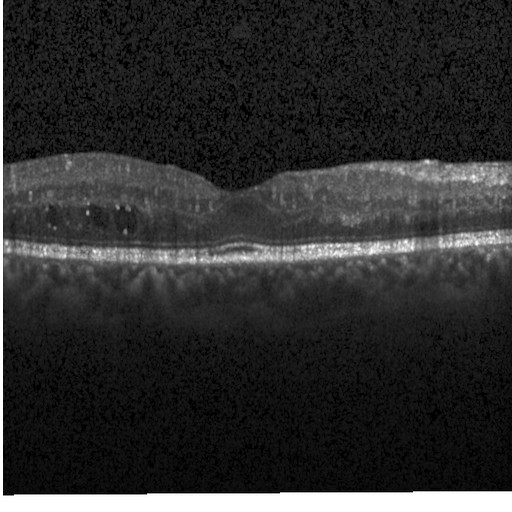
Horizontal scan through the fovea; retinal OCT cross-section; spectral-domain optical coherence tomography; Heidelberg Spectralis. Finding: DME.